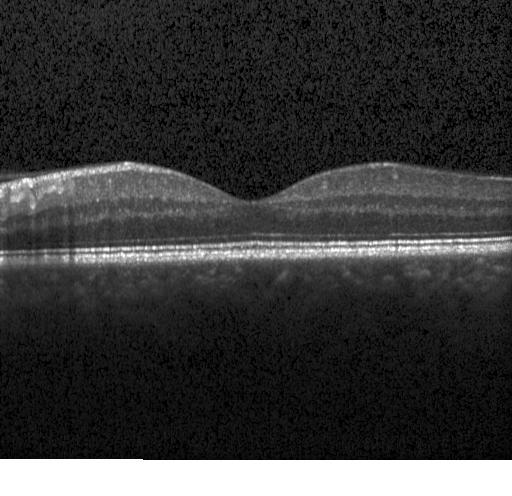
Finding: no evidence of choroidal neovascularization, diabetic macular edema, or drusen.